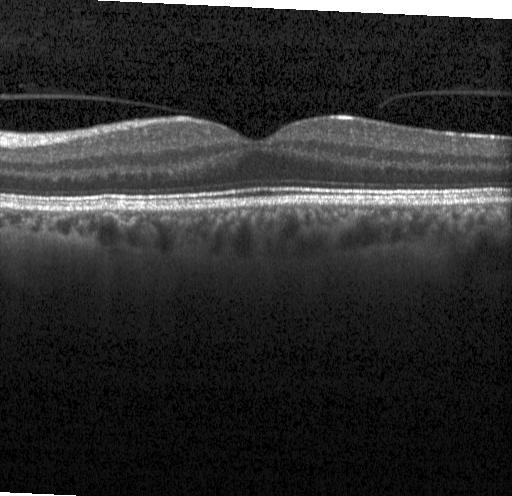 Optical coherence tomography B-scan, acquired on a Heidelberg Spectralis, centered on the fovea, spectral-domain OCT.
Impression: no choroidal neovascularization, no diabetic macular edema, and no drusen.